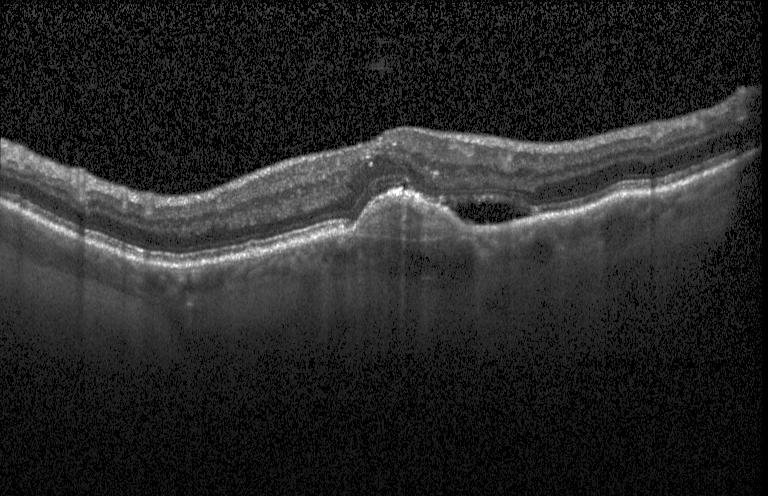
Optical coherence tomography scan, instrument: Heidelberg Spectralis. This B-scan demonstrates choroidal neovascularization.